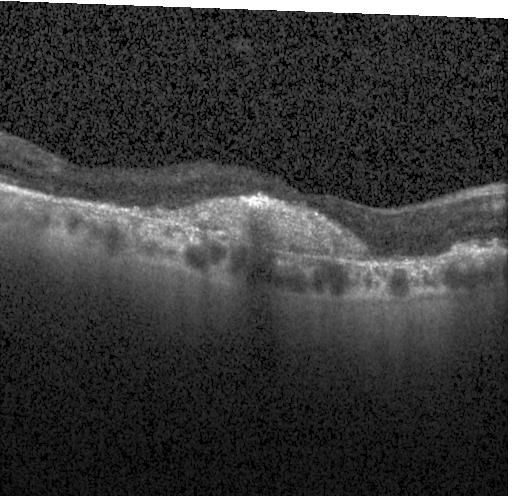
Impression: choroidal neovascularization.